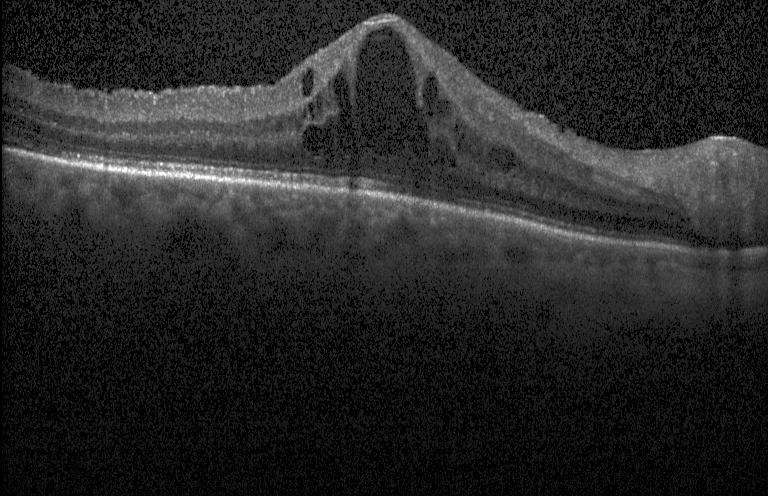 Optical coherence tomography B-scan · horizontal scan through the fovea · spectral-domain OCT · instrument: Heidelberg Spectralis — OCT finding: diabetic macular edema (DME).